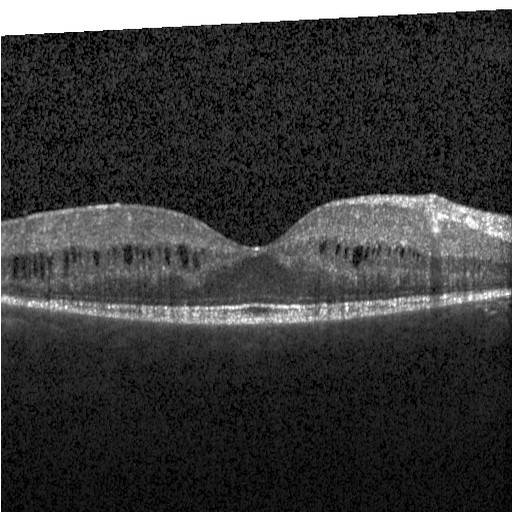

Fovea-centered; OCT B-scan. This B-scan demonstrates diabetic macular edema (DME).